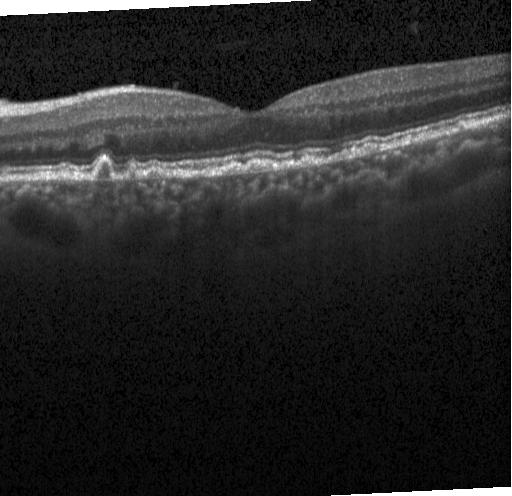
The scan shows multiple drusen.